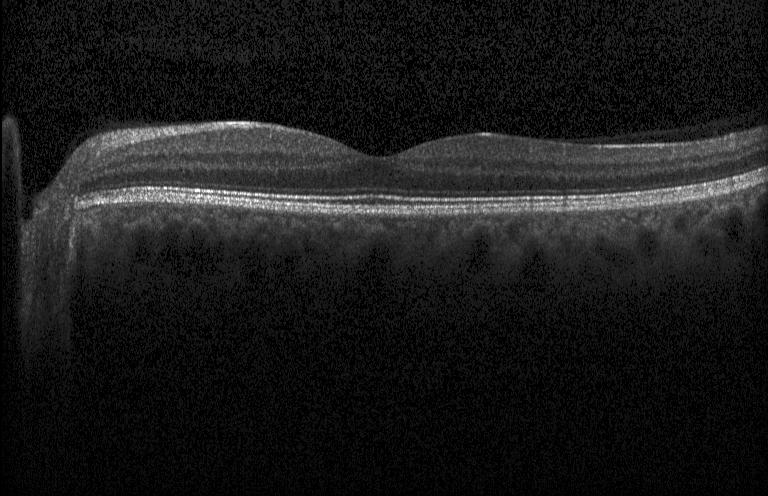
Impression: no choroidal neovascularization, no diabetic macular edema, and no drusen.